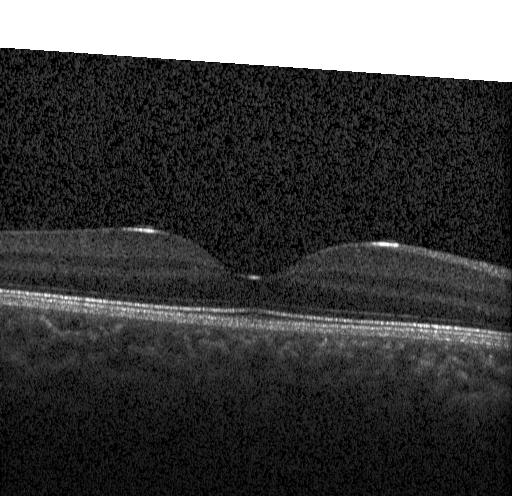

Retinal OCT B-scan, acquired on a Heidelberg Spectralis. Impression: no choroidal neovascularization, diabetic macular edema, or drusen.